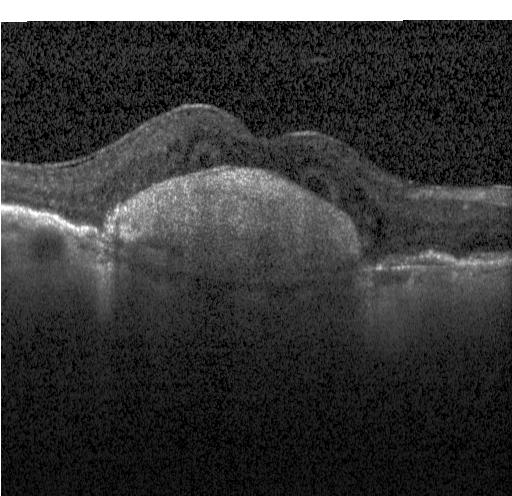

OCT finding: a choroidal neovascular membrane.